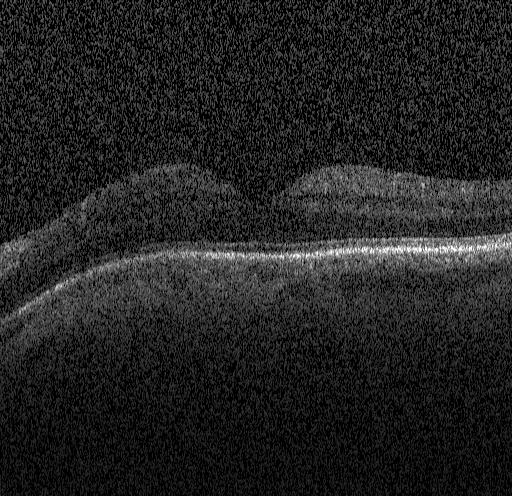
OCT B-scan showing neither CNV, DME, nor drusen.